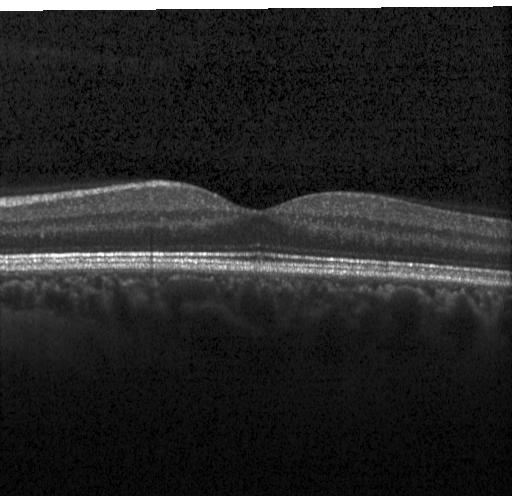
Spectral-domain optical coherence tomography, retinal OCT cross-section, through the macula — Finding: no evidence of choroidal neovascularization, diabetic macular edema, or drusen.